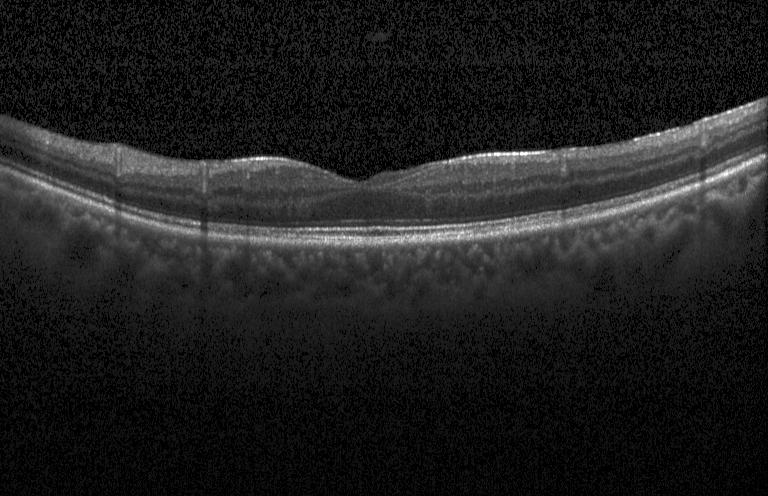 Macular OCT: no evidence of CNV, DME, or drusen.